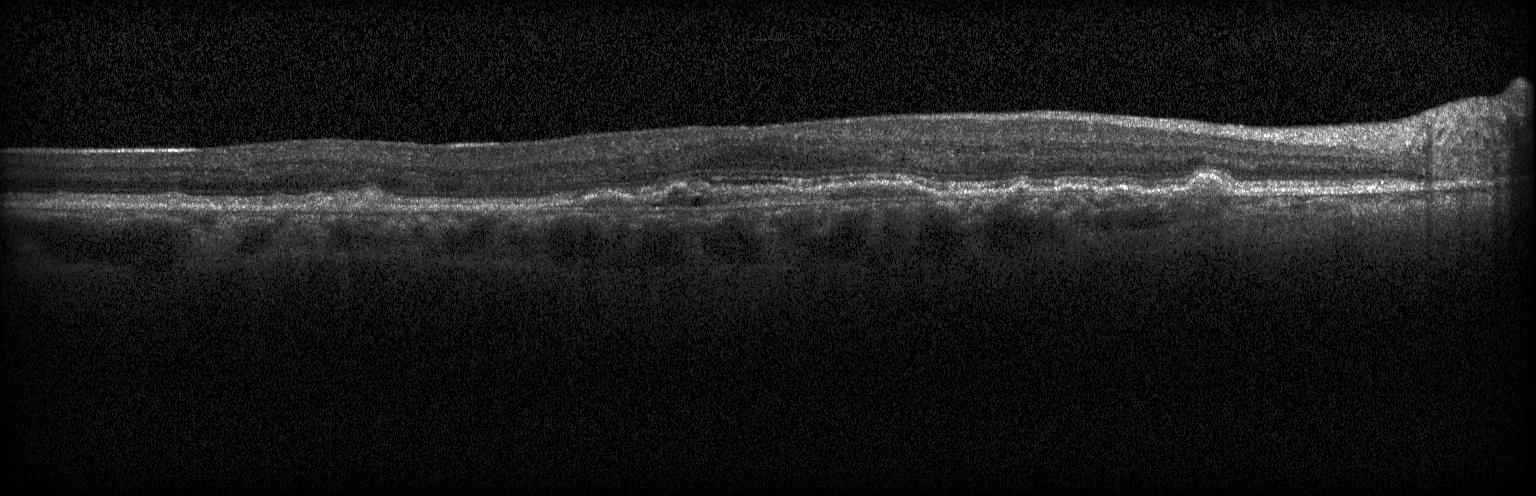 This B-scan demonstrates a choroidal neovascular membrane.